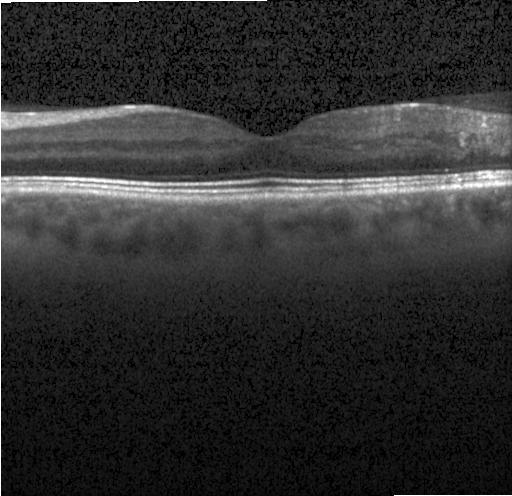
Macular OCT demonstrating no CNV, no DME, and no drusen.